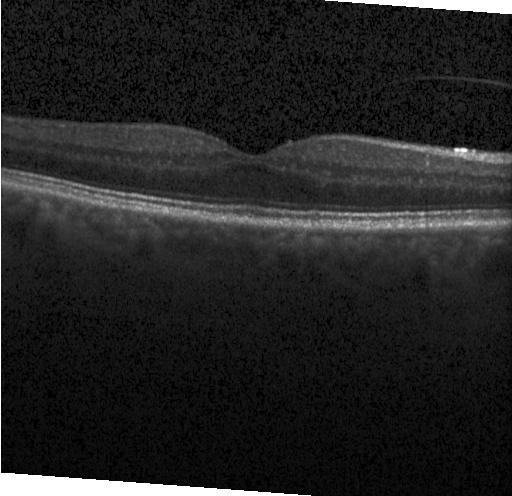 Macular scan · SD-OCT · optical coherence tomography B-scan.
Diagnosis: neither choroidal neovascularization, diabetic macular edema, nor drusen.